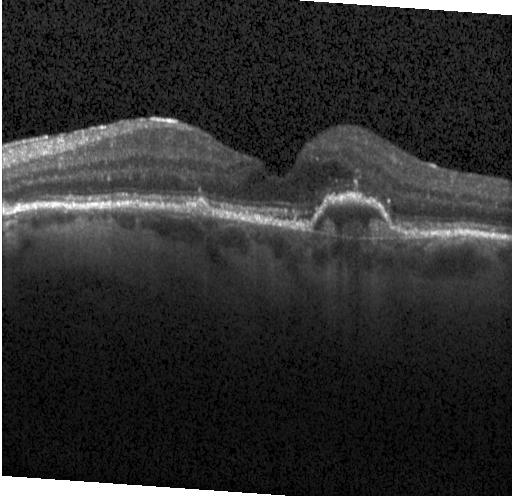

OCT line scan.
Finding: CNV.